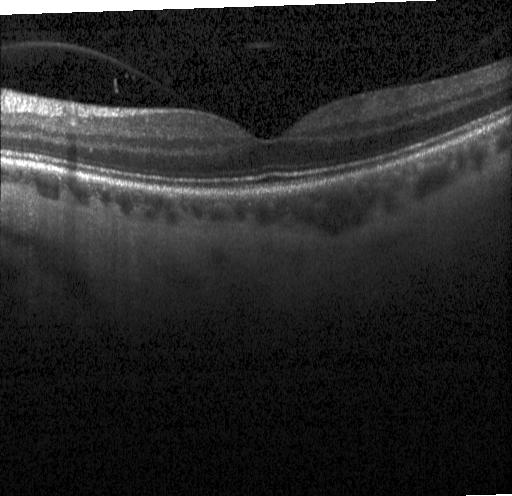

SD-OCT; OCT B-scan; centered on the fovea; instrument: Heidelberg Spectralis — Impression: no choroidal neovascularization, no diabetic macular edema, and no drusen.